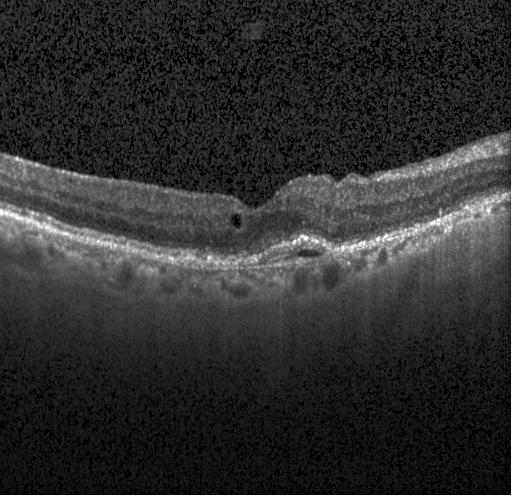
OCT line scan, macular scan
OCT finding: a choroidal neovascular membrane.